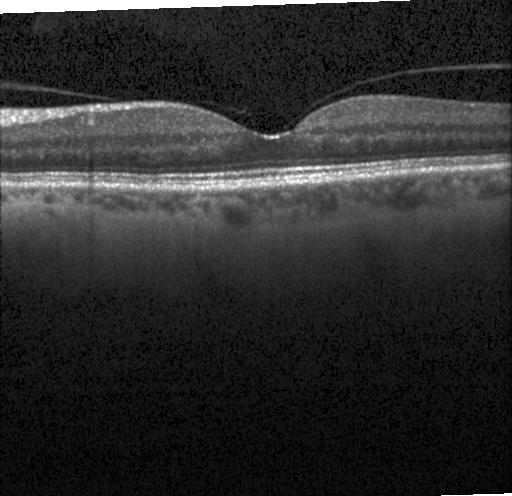

Centered on the fovea, retinal OCT B-scan. No CNV, no DME, and no drusen.